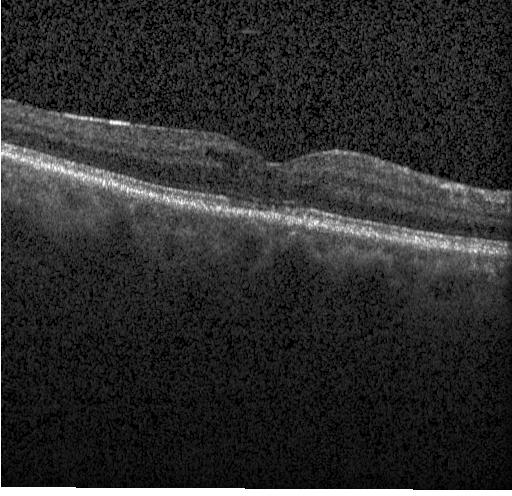
Acquired on a Heidelberg Spectralis · optical coherence tomography scan.
Impression: diabetic macular edema.